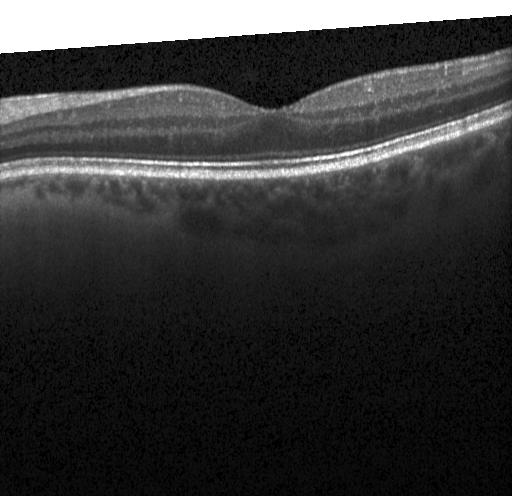 OCT finding: no evidence of choroidal neovascularization, diabetic macular edema, or drusen.